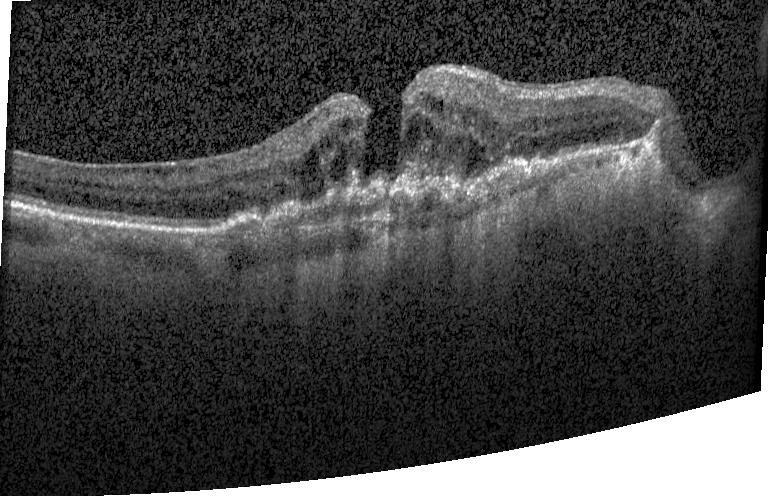
OCT finding: choroidal neovascularization (CNV).